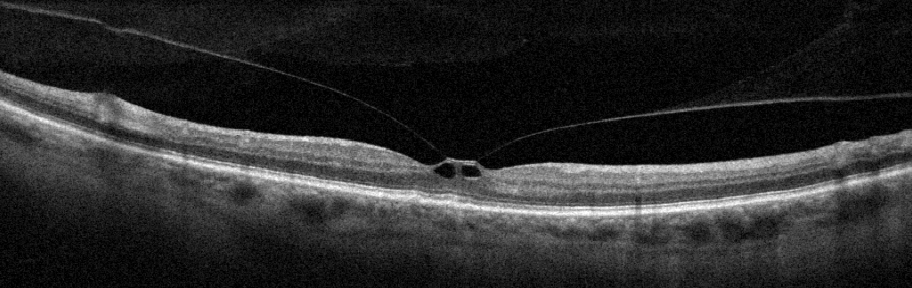
Spectral-domain OCT B-scan: vitreomacular interface disease.